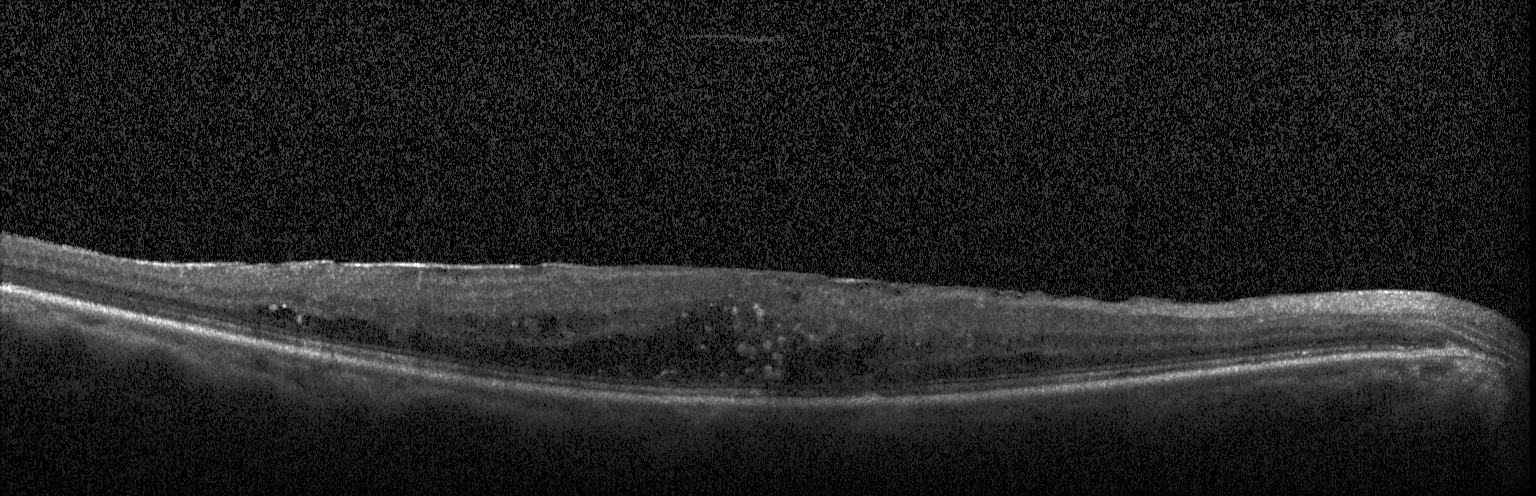
OCT B-scan — This B-scan demonstrates DME.